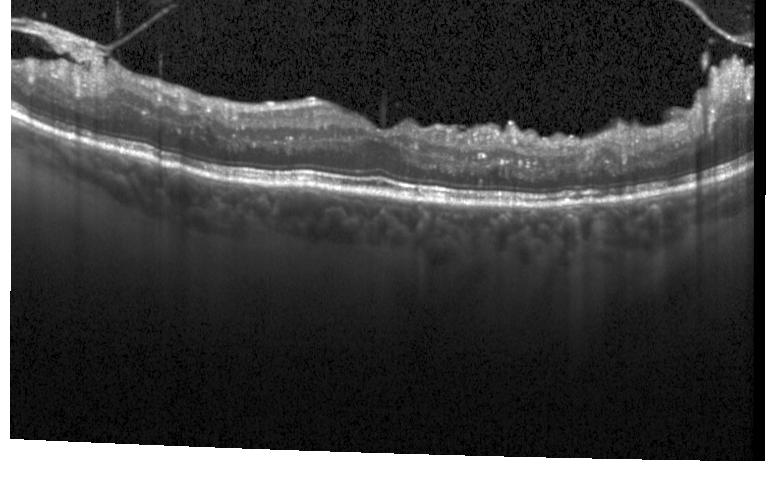 This B-scan demonstrates DME.